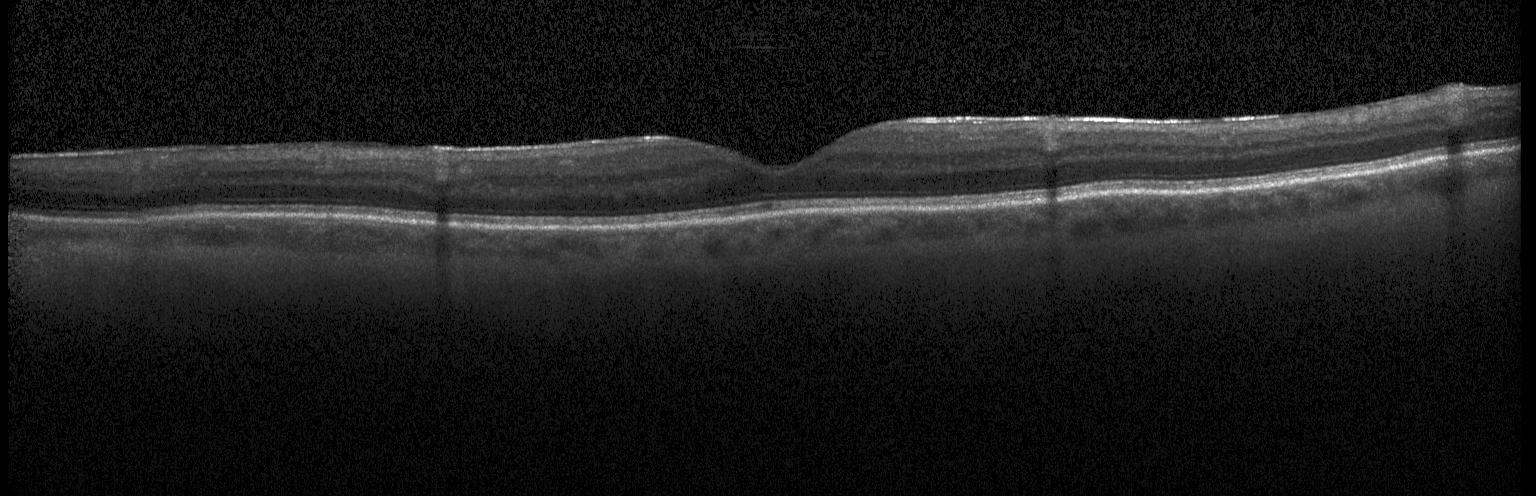
Through the macula; retinal OCT B-scan; spectral-domain OCT — Neither CNV, DME, nor drusen.